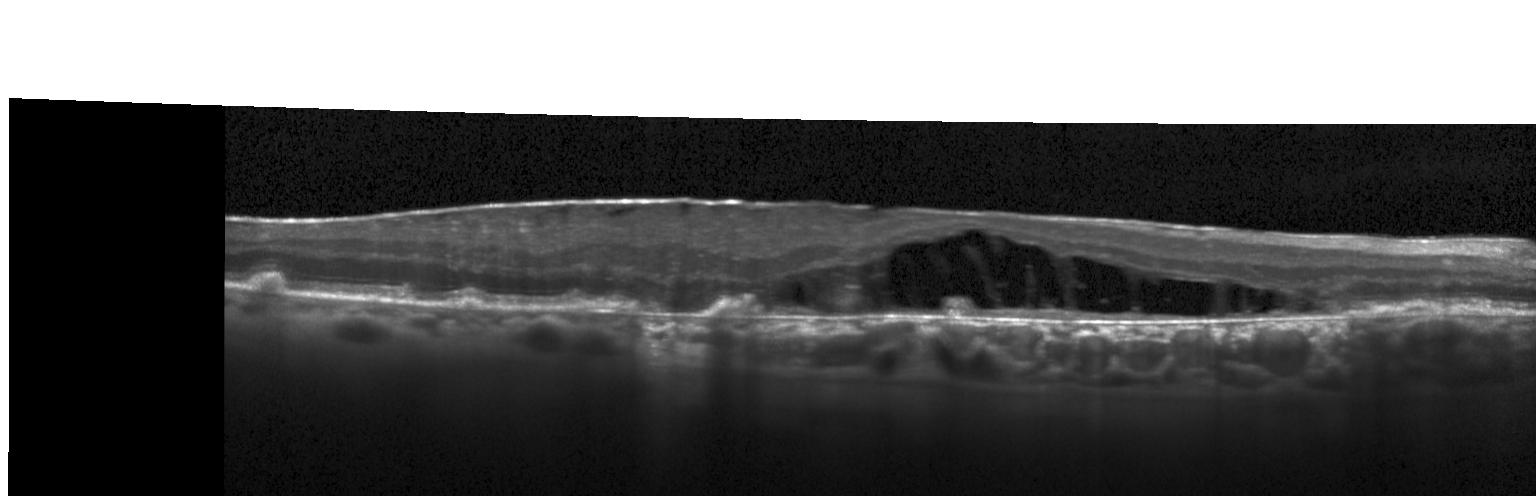 SD-OCT, instrument: Heidelberg Spectralis, retinal OCT B-scan. Impression: choroidal neovascularization (CNV).